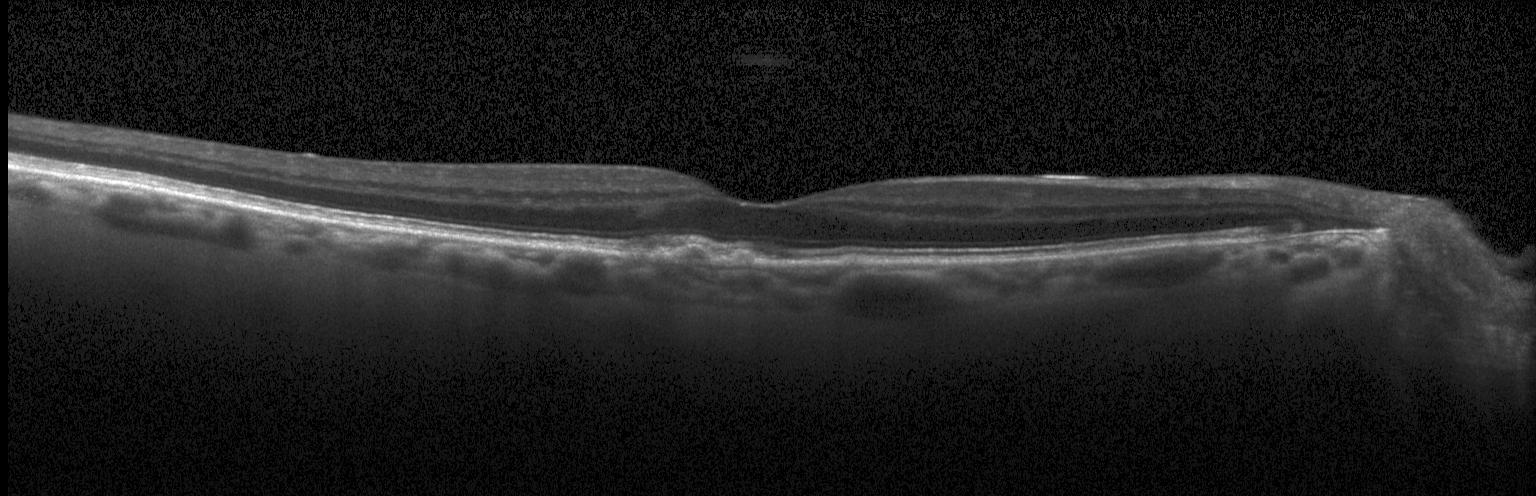 Retinal OCT B-scan, horizontal scan through the fovea.
Assessment: drusen.